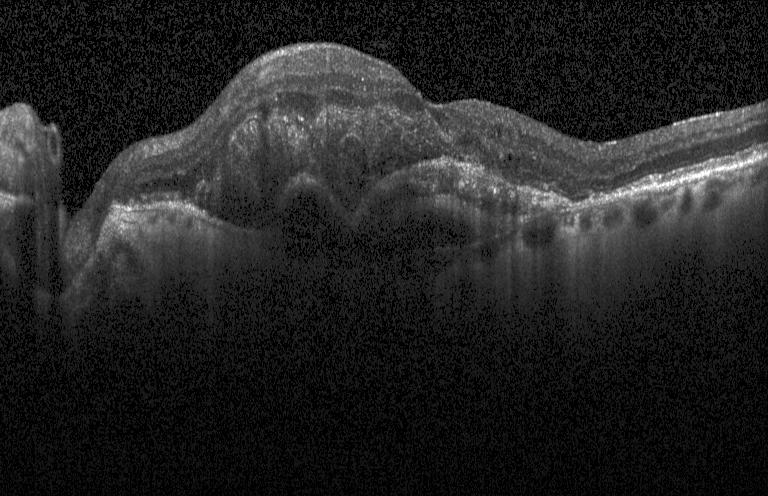 Macular OCT: a choroidal neovascular membrane.